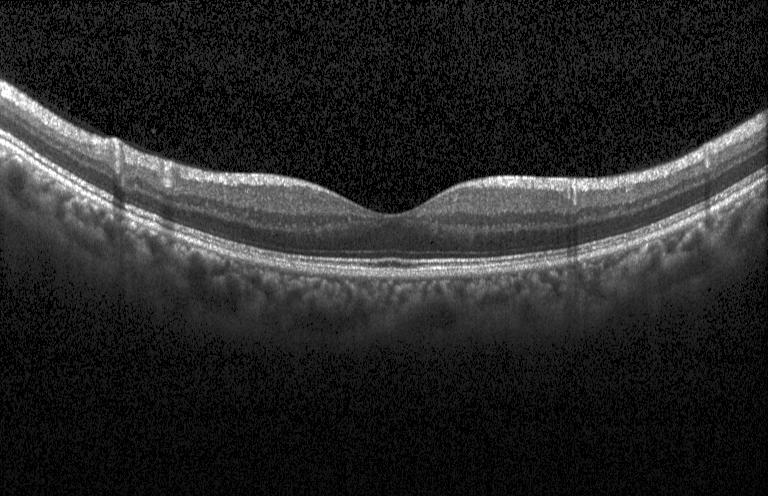

Spectral-domain optical coherence tomography, horizontal scan through the fovea, optical coherence tomography scan, Heidelberg Spectralis OCT system — Finding: no evidence of choroidal neovascularization, diabetic macular edema, or drusen.